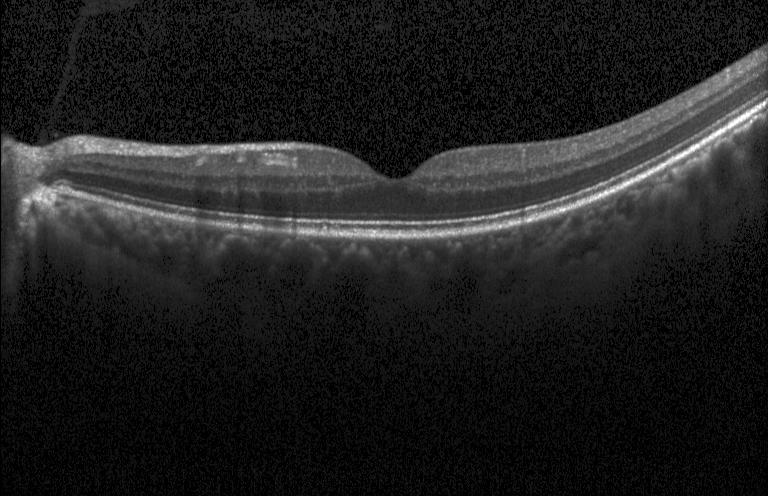 Retinal OCT cross-section.
Finding: no choroidal neovascularization, no diabetic macular edema, and no drusen.